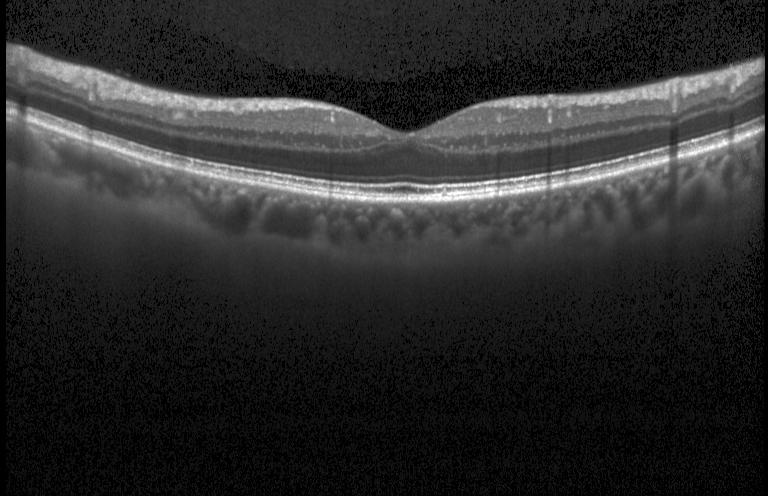

SD-OCT · retinal OCT cross-section. This B-scan demonstrates no evidence of CNV, DME, or drusen.